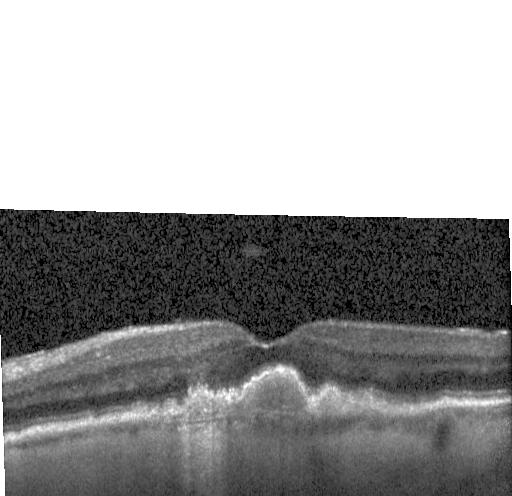 Spectral-domain optical coherence tomography, optical coherence tomography scan — Assessment: a choroidal neovascular membrane.